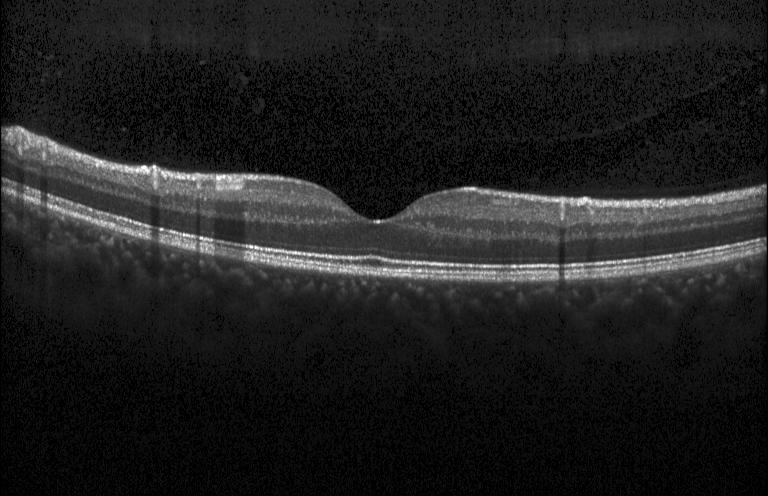

Retinal OCT cross-section. Heidelberg Spectralis. Spectral-domain optical coherence tomography — Impression: no choroidal neovascularization, diabetic macular edema, or drusen.